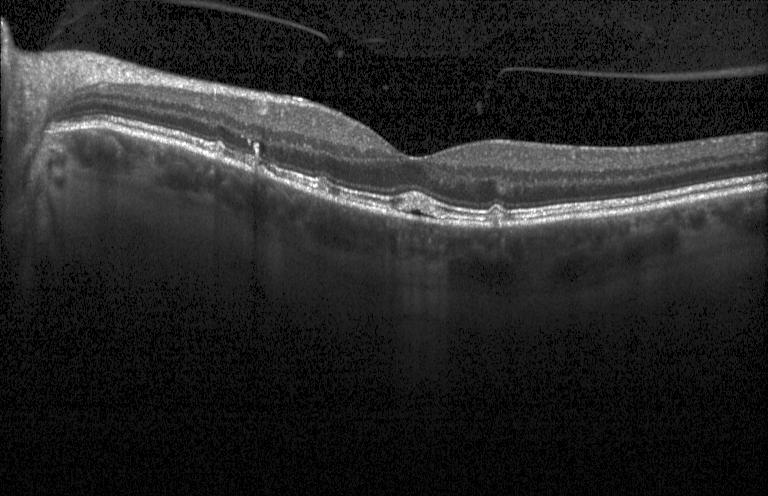 Finding: multiple drusen.